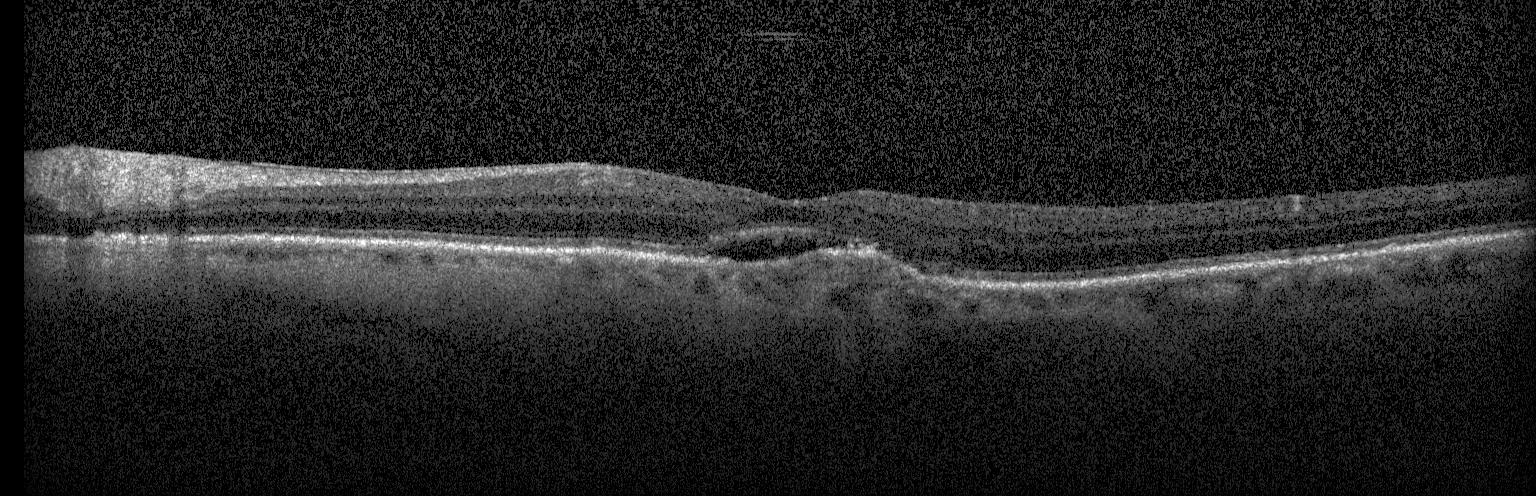
Finding: CNV.